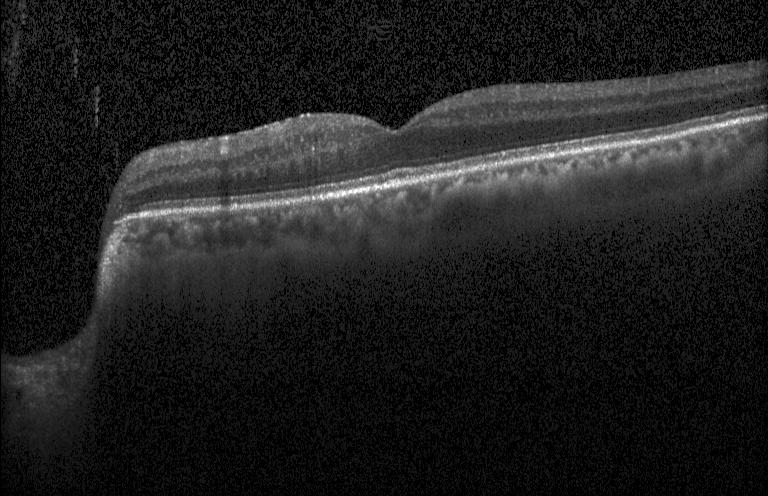 SD-OCT; optical coherence tomography scan
Dx: no evidence of CNV, DME, or drusen.